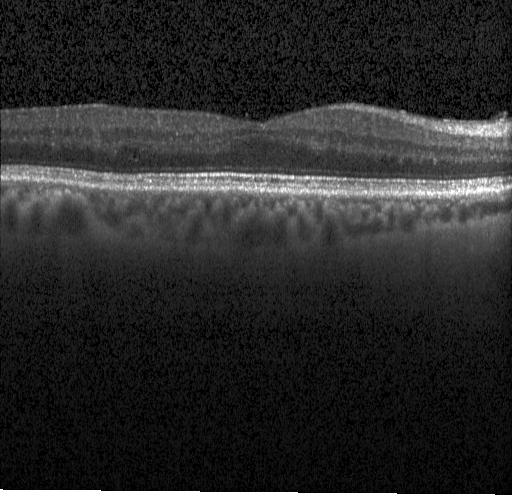
Diagnosis: neither choroidal neovascularization, diabetic macular edema, nor drusen.